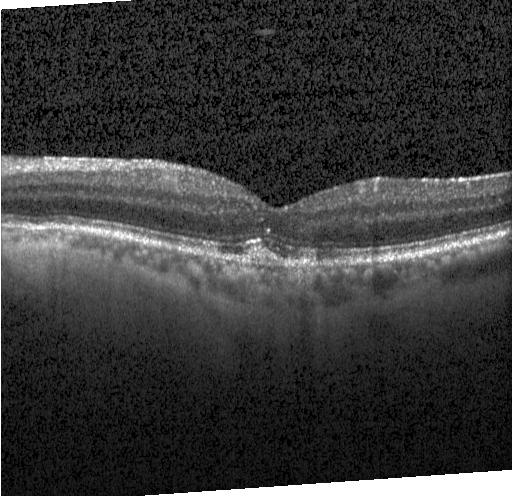 Retinal OCT B-scan; through the macula; instrument: Heidelberg Spectralis; spectral-domain optical coherence tomography — The scan shows choroidal neovascularization (CNV).